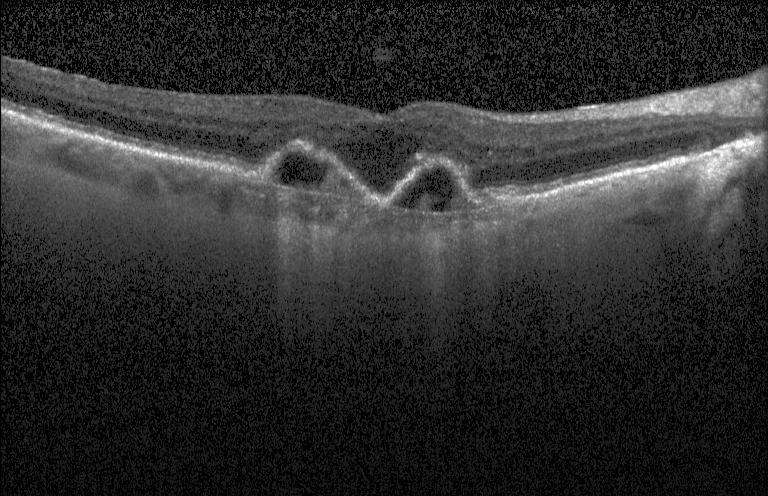
Optical coherence tomography B-scan · SD-OCT · Heidelberg Spectralis
Macular OCT: CNV.